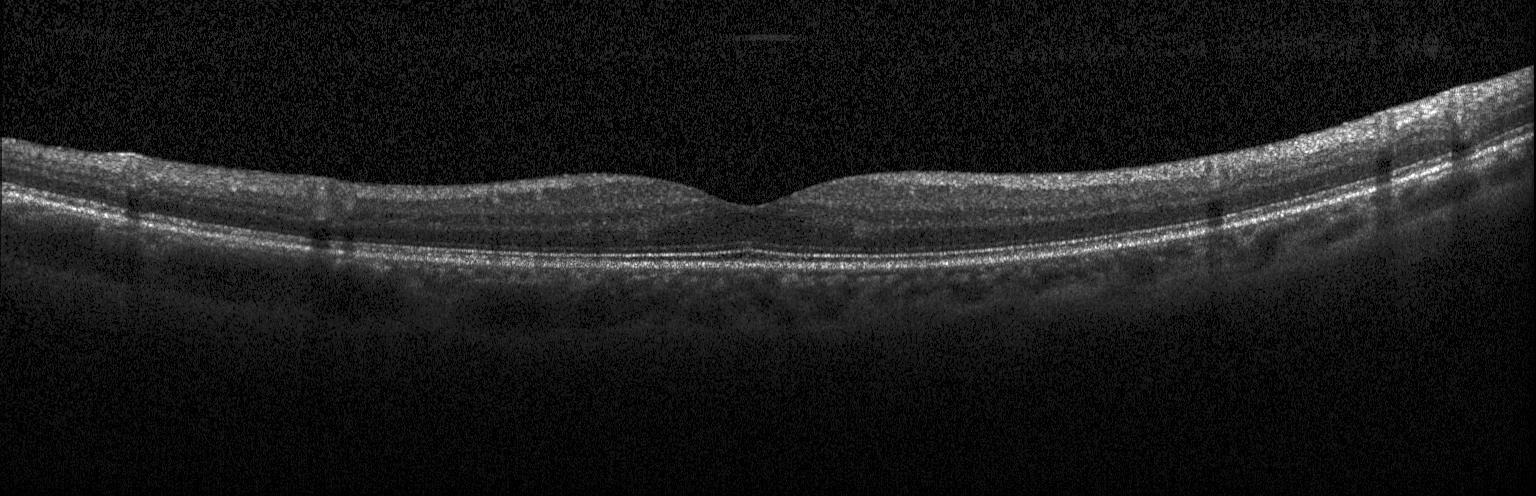

Finding: no choroidal neovascularization, diabetic macular edema, or drusen.